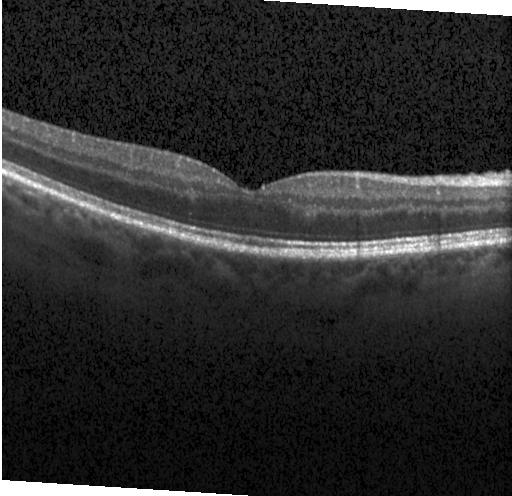

Optical coherence tomography scan · horizontal scan through the fovea. Diagnosis: no choroidal neovascularization, no diabetic macular edema, and no drusen.